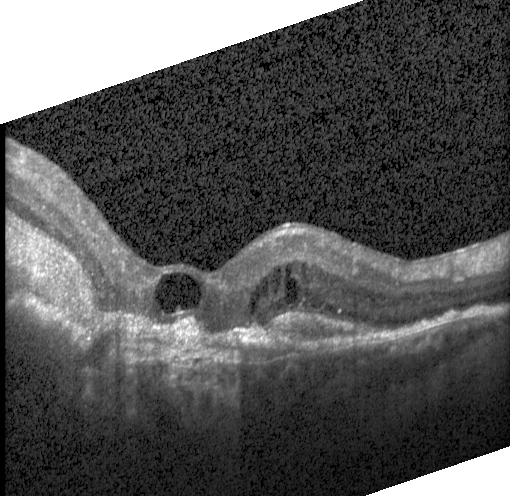

Retinal OCT cross-section — Finding: choroidal neovascularization.